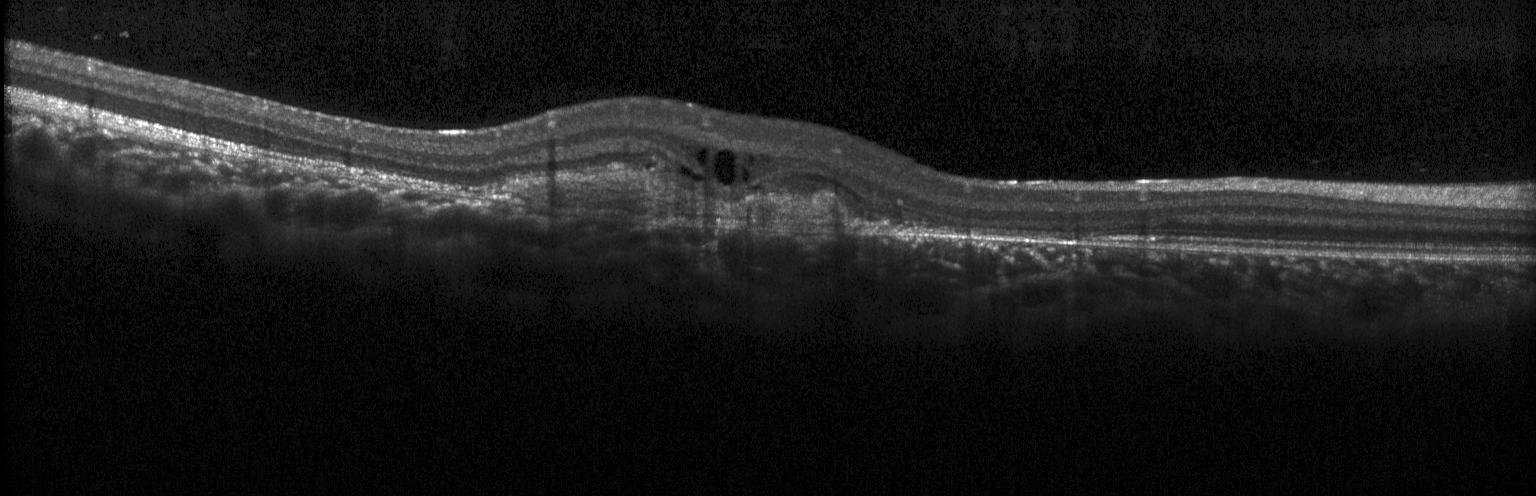

Instrument: Heidelberg Spectralis. OCT line scan — OCT finding: a choroidal neovascular membrane.